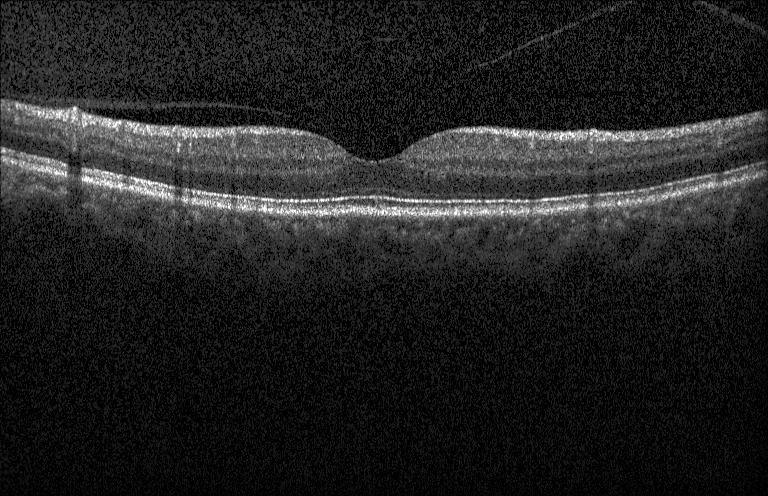

Spectral-domain OCT B-scan: no choroidal neovascularization, no diabetic macular edema, and no drusen.